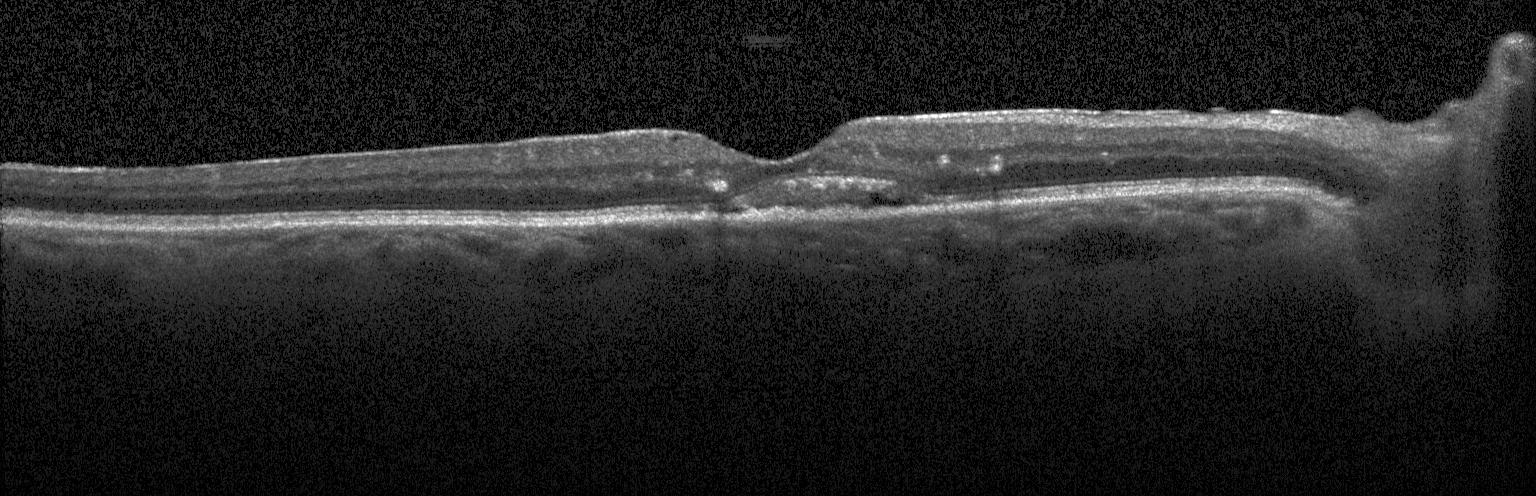
Diagnosis: choroidal neovascularization (CNV).